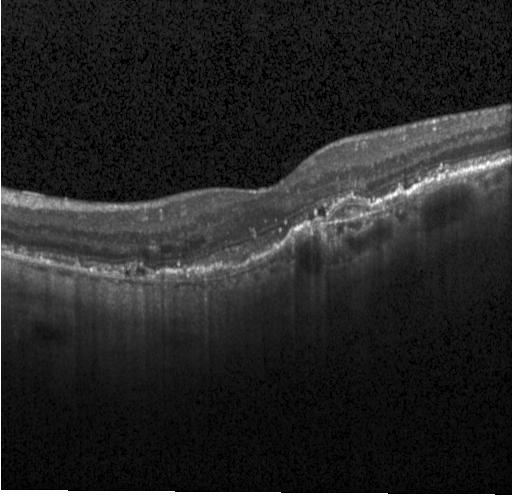 Spectral-domain OCT, horizontal scan through the fovea, retinal OCT B-scan, acquired on a Heidelberg Spectralis.
Macular OCT: a choroidal neovascular membrane.